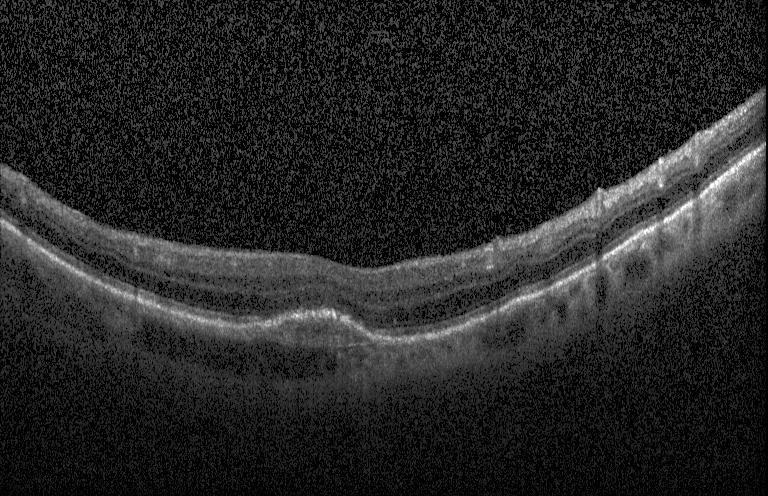
Retinal OCT B-scan. Acquired on a Heidelberg Spectralis. Macular OCT: CNV.